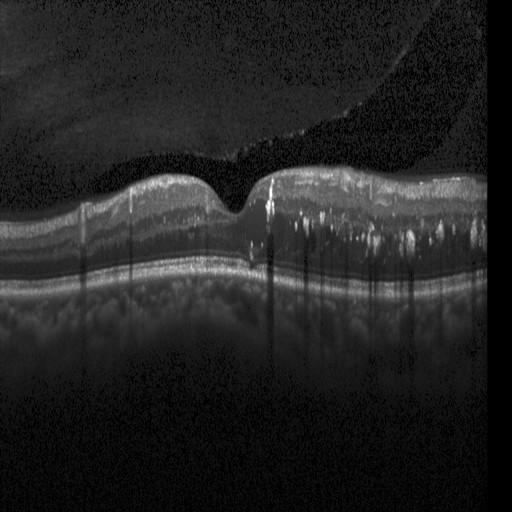

Optical coherence tomography scan — Finding: DME.